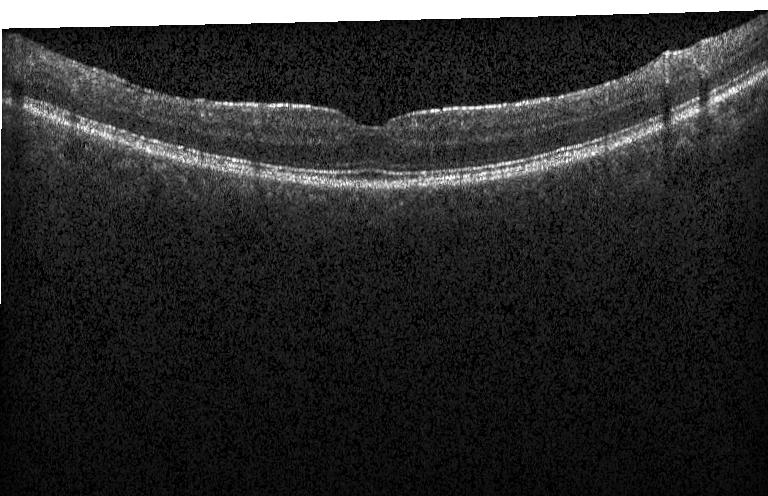 Optical coherence tomography B-scan · horizontal scan through the fovea · acquired on a Heidelberg Spectralis
The scan shows no evidence of choroidal neovascularization, diabetic macular edema, or drusen.